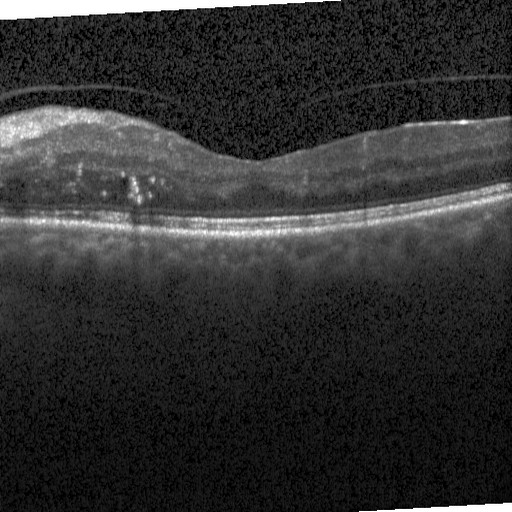

Retinal OCT cross-section showing diabetic macular edema.